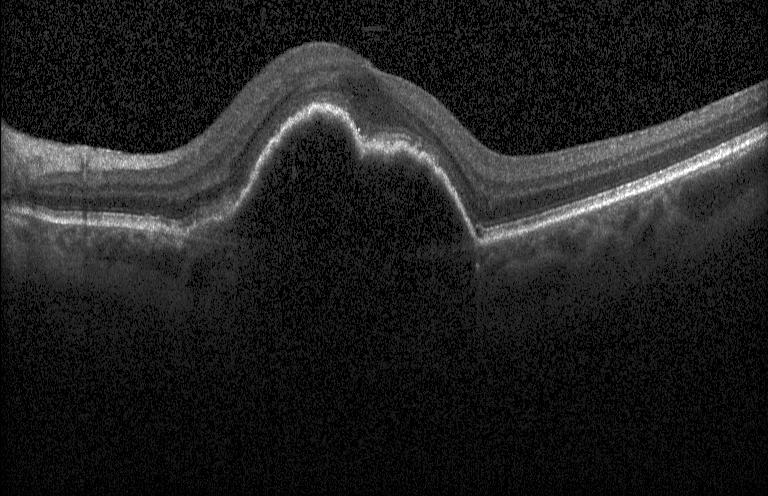

Macular scan; Heidelberg Spectralis OCT system; retinal OCT cross-section. Impression: a choroidal neovascular membrane.